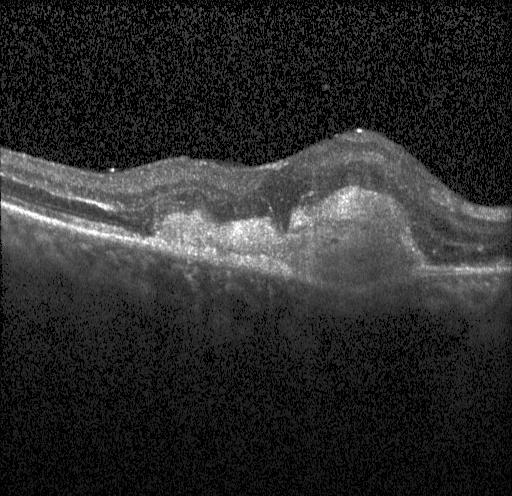
Retinal OCT cross-section, spectral-domain optical coherence tomography. The scan shows a choroidal neovascular membrane.